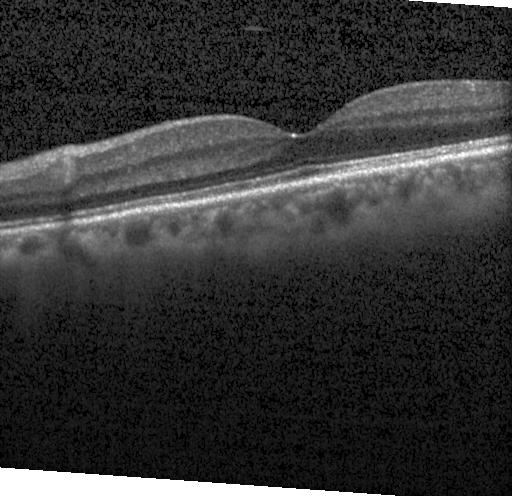 SD-OCT; OCT B-scan
Diagnosis: no evidence of CNV, DME, or drusen.